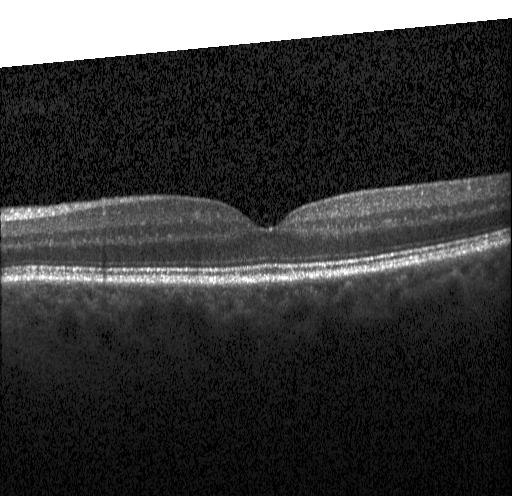
Optical coherence tomography scan. Instrument: Heidelberg Spectralis.
This B-scan demonstrates no evidence of CNV, DME, or drusen.